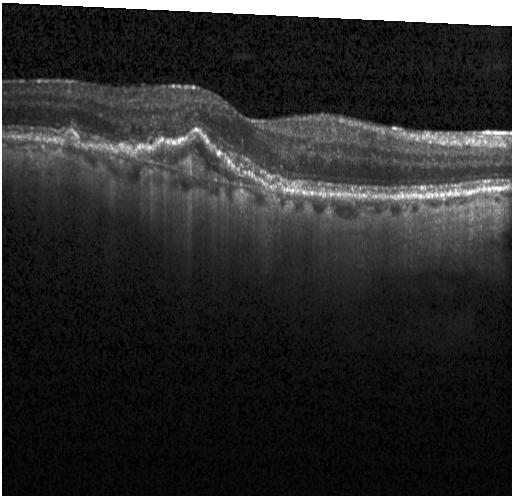

Spectral-domain optical coherence tomography · acquired on a Heidelberg Spectralis · macular scan · retinal OCT B-scan
Impression: a choroidal neovascular membrane.